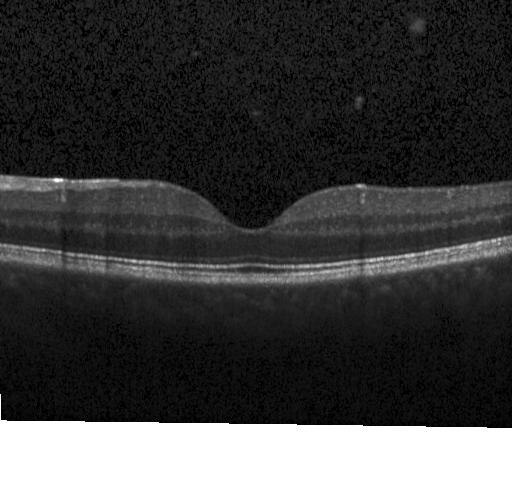
Macular scan, OCT B-scan. No choroidal neovascularization, diabetic macular edema, or drusen.